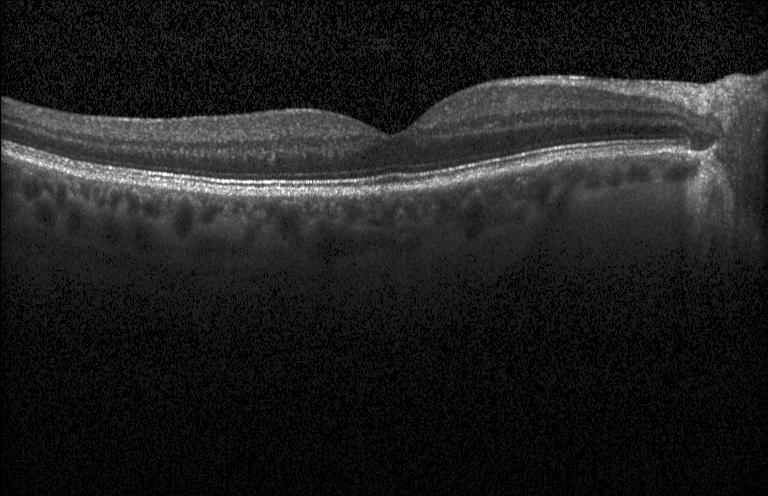 OCT B-scan — This B-scan demonstrates neither choroidal neovascularization, diabetic macular edema, nor drusen.